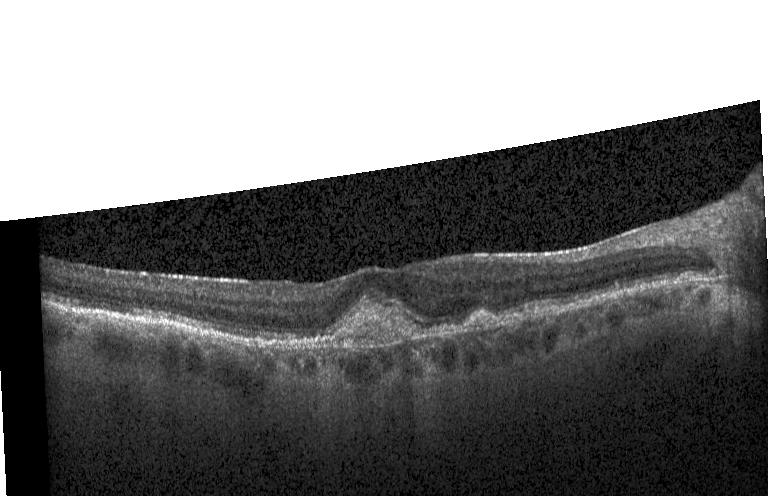
OCT line scan — OCT finding: a choroidal neovascular membrane.